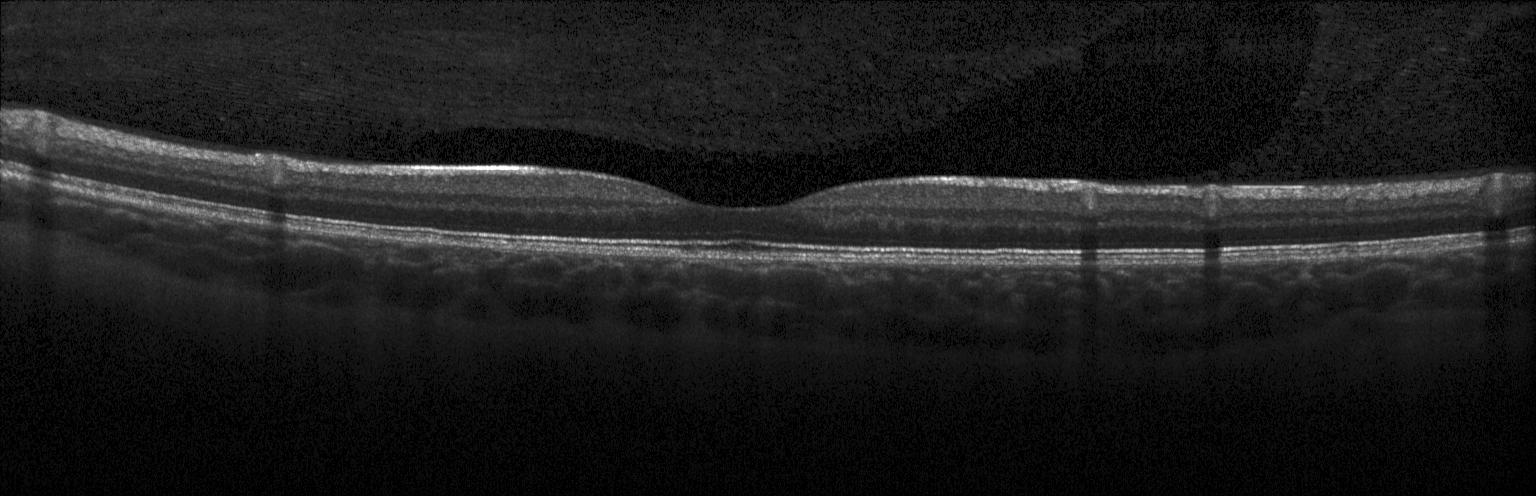 Retinal OCT cross-section · instrument: Heidelberg Spectralis. Dx: neither choroidal neovascularization, diabetic macular edema, nor drusen.